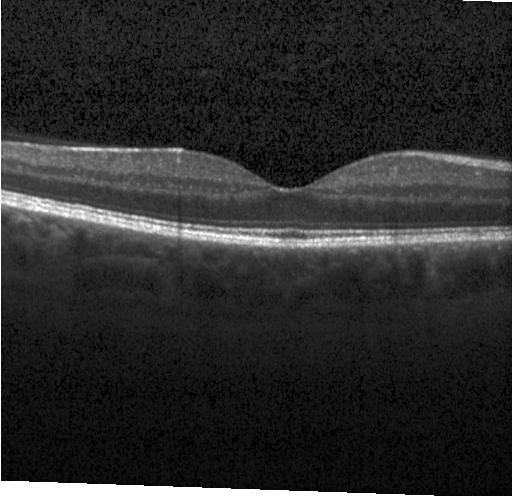 Retinal OCT B-scan. Through the macula. SD-OCT
No choroidal neovascularization, diabetic macular edema, or drusen.